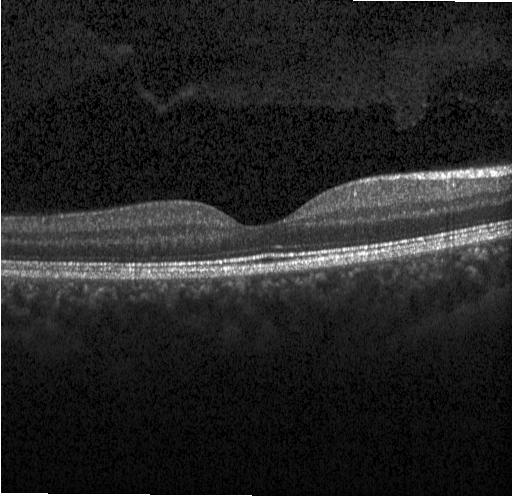

Heidelberg Spectralis · OCT B-scan · spectral-domain optical coherence tomography · macular scan
Finding: neither CNV, DME, nor drusen.